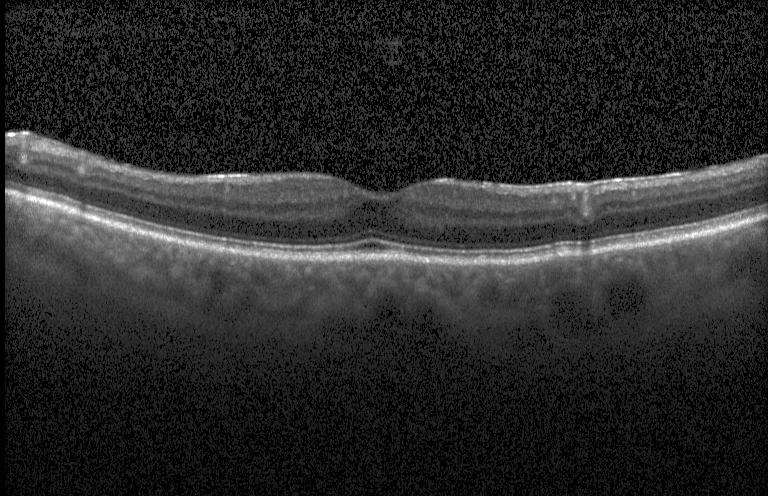 Finding: no choroidal neovascularization, diabetic macular edema, or drusen.